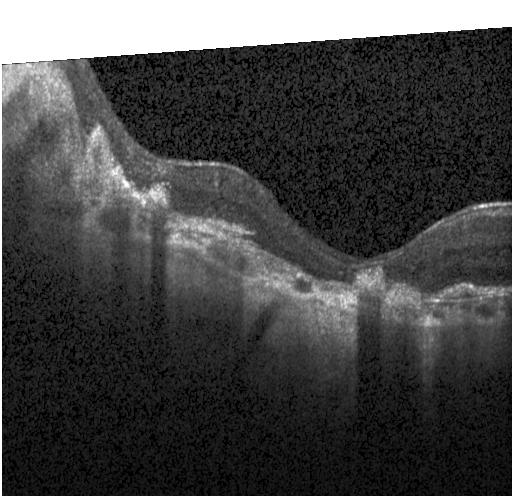 Retinal OCT cross-section
OCT finding: a choroidal neovascular membrane.